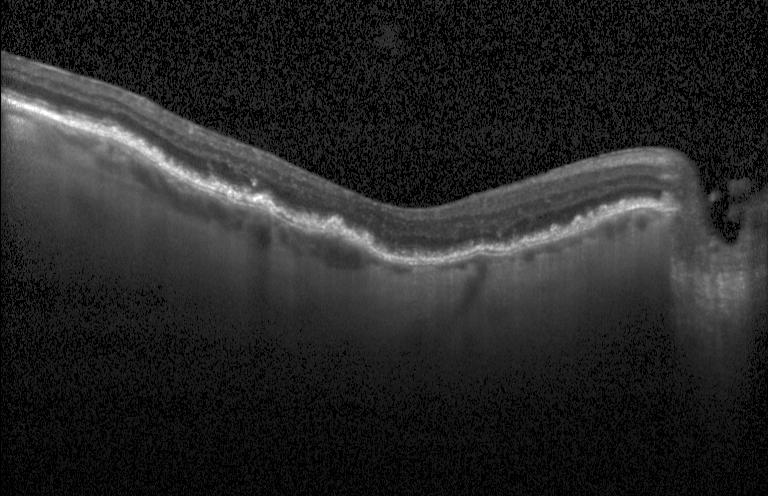
Finding: a choroidal neovascular membrane.